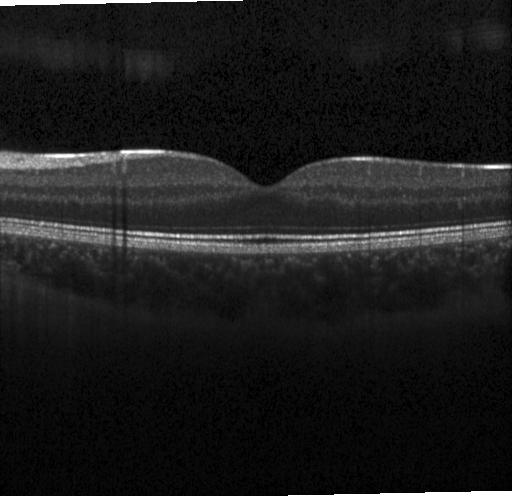

OCT finding: no CNV, no DME, and no drusen.